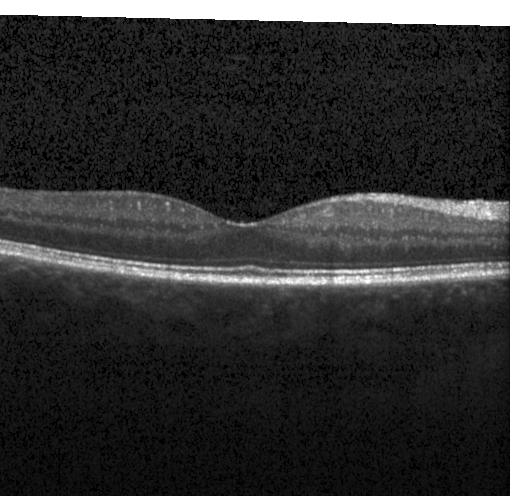 This B-scan demonstrates no CNV, DME, or drusen.